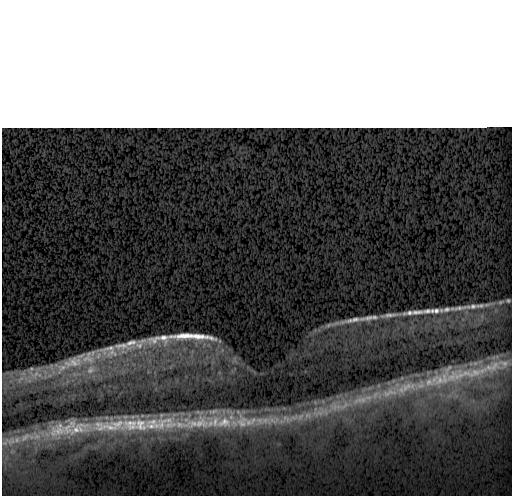

Optical coherence tomography scan — Impression: no CNV, no DME, and no drusen.